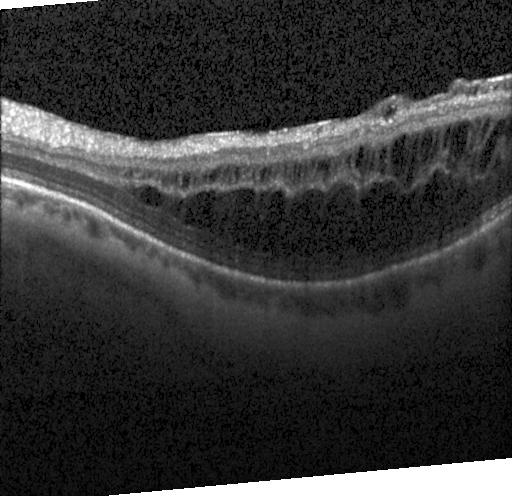
Retinal OCT cross-section showing diabetic macular edema.